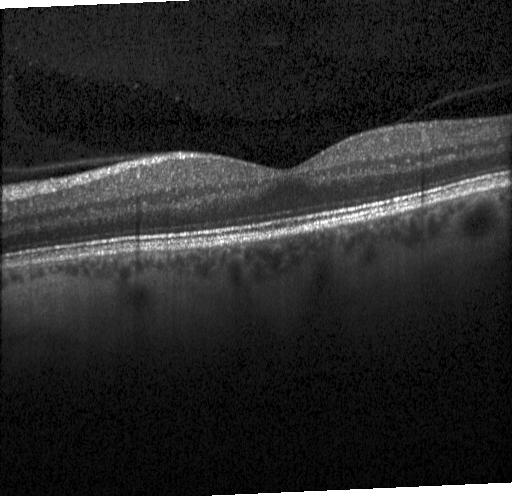

Retinal OCT cross-section.
Diagnosis: no choroidal neovascularization, no diabetic macular edema, and no drusen.